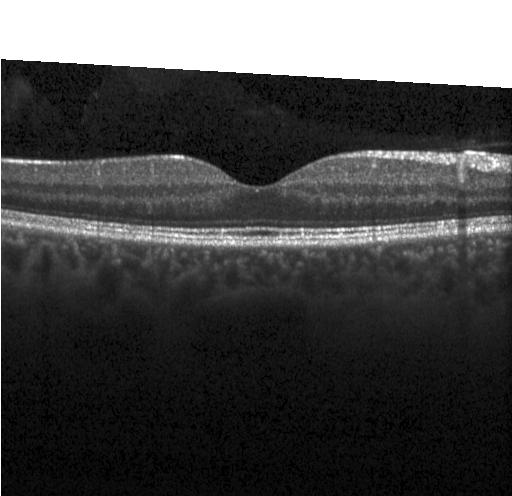 The scan shows no evidence of choroidal neovascularization, diabetic macular edema, or drusen.